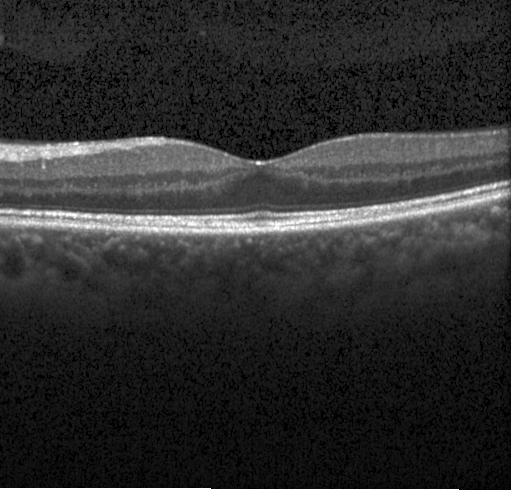

Centered on the fovea, OCT B-scan, SD-OCT
Impression: neither CNV, DME, nor drusen.